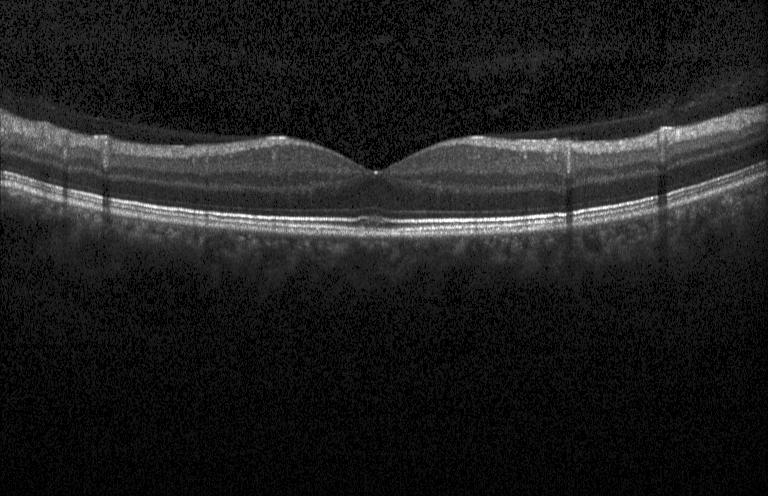 Heidelberg Spectralis OCT system, centered on the fovea, OCT B-scan. The scan shows no evidence of CNV, DME, or drusen.